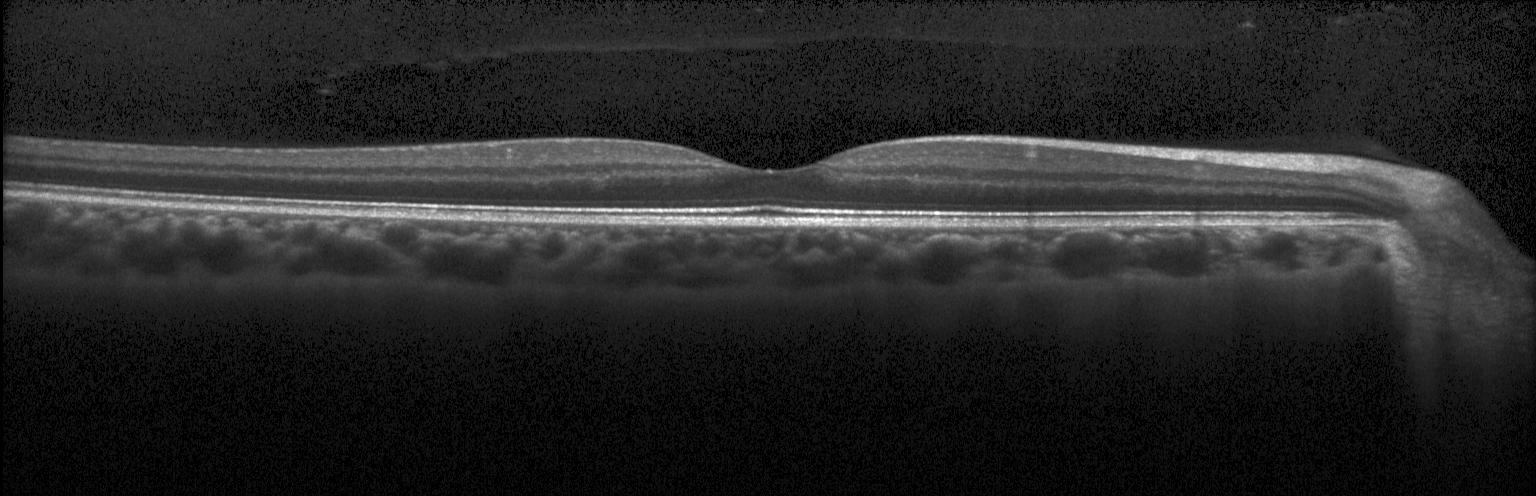
This B-scan demonstrates no choroidal neovascularization, no diabetic macular edema, and no drusen.